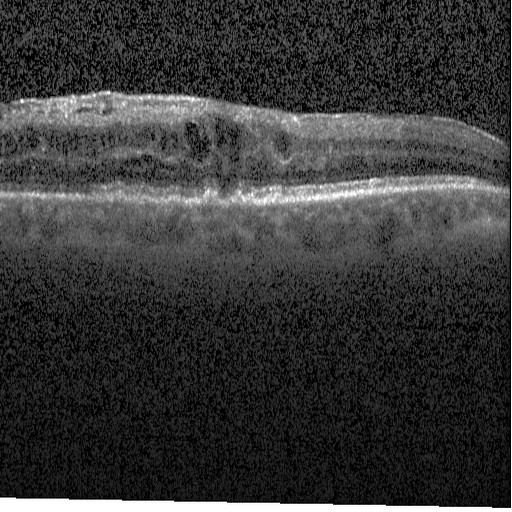
Spectral-domain optical coherence tomography. Retinal OCT cross-section. Through the macula. Heidelberg Spectralis.
Macular OCT: diabetic macular edema.